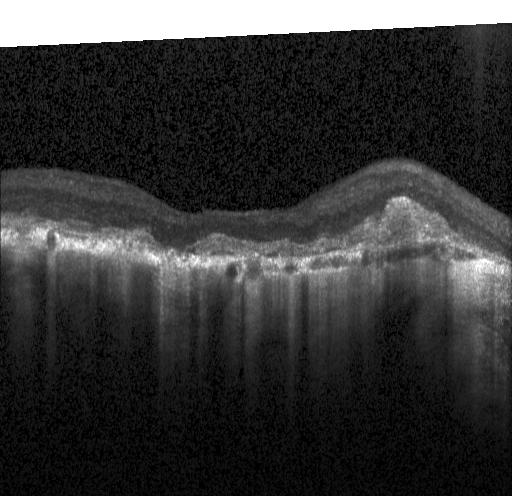

OCT line scan, Heidelberg Spectralis OCT system, SD-OCT, macular scan. Macular OCT: a choroidal neovascular membrane.